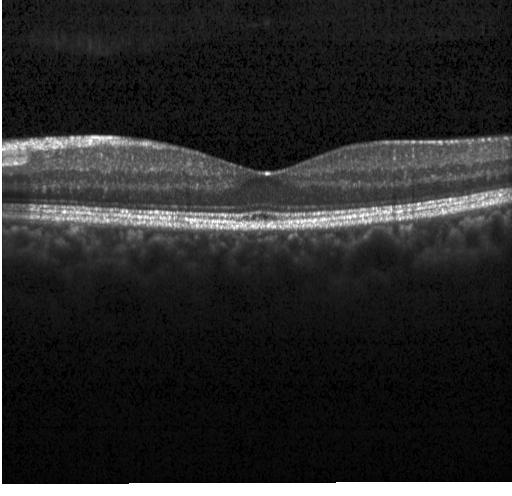

OCT B-scan showing no evidence of CNV, DME, or drusen.